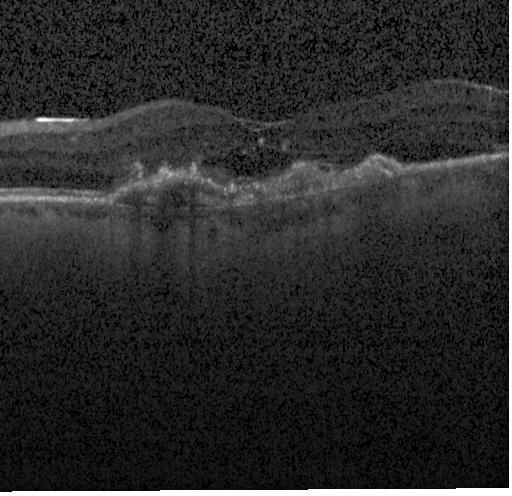
OCT B-scan
Dx: a choroidal neovascular membrane.